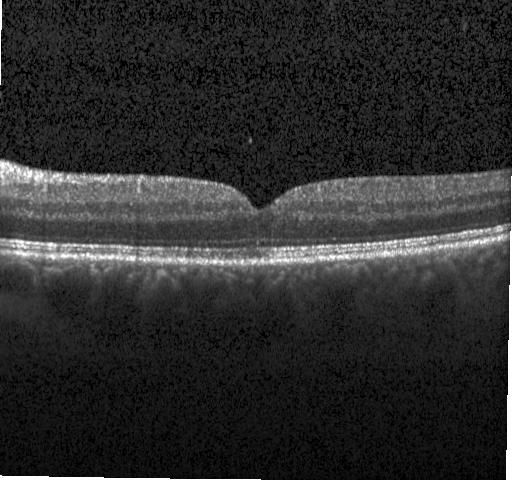

Heidelberg Spectralis OCT system. Macular scan. Optical coherence tomography scan. SD-OCT. Diagnosis: no evidence of CNV, DME, or drusen.